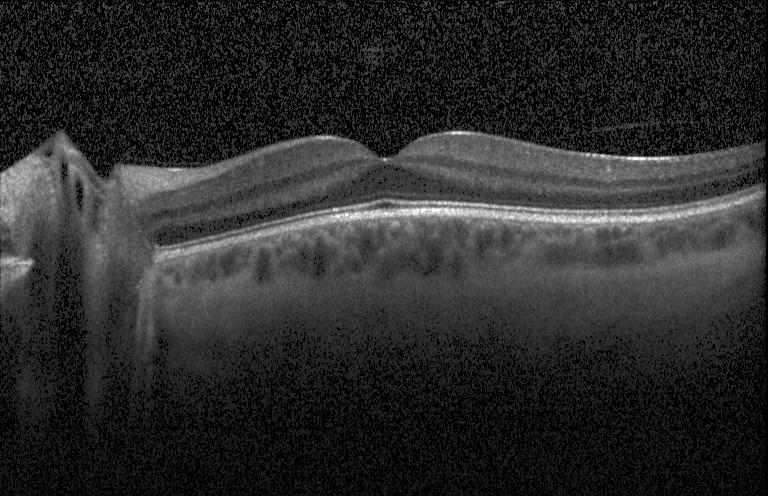

SD-OCT · optical coherence tomography B-scan · Heidelberg Spectralis.
This B-scan demonstrates no choroidal neovascularization, no diabetic macular edema, and no drusen.